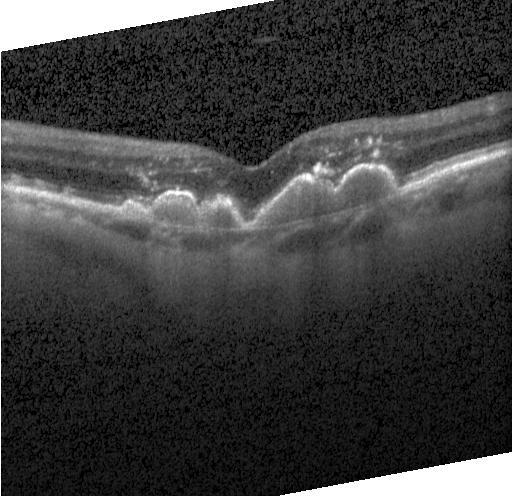 Optical coherence tomography scan
Diagnosis: choroidal neovascularization.